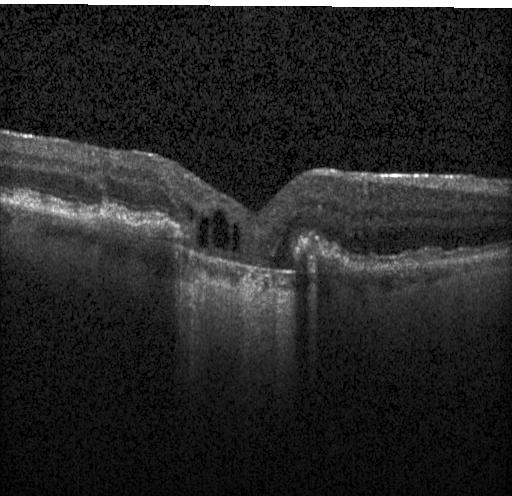

Macular OCT: choroidal neovascularization.